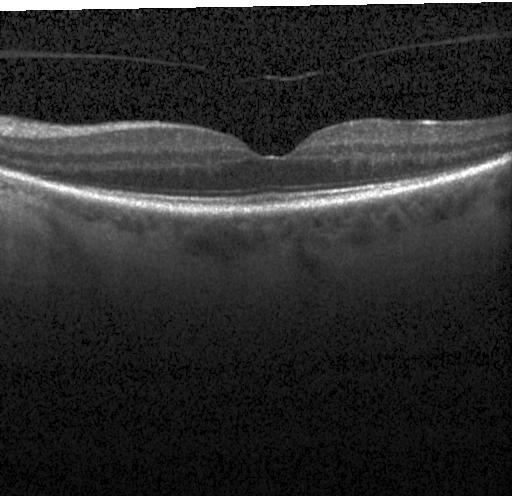
Spectral-domain optical coherence tomography. Optical coherence tomography B-scan. Centered on the fovea — Dx: neither choroidal neovascularization, diabetic macular edema, nor drusen.